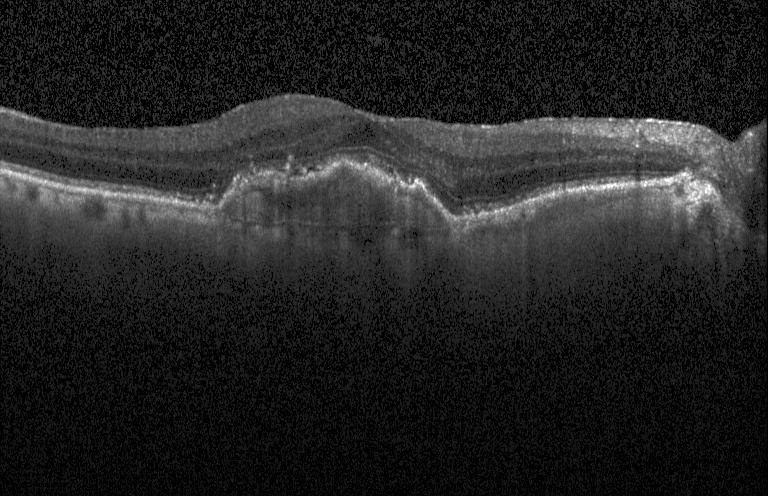

Acquired on a Heidelberg Spectralis; OCT line scan.
Dx: choroidal neovascularization.